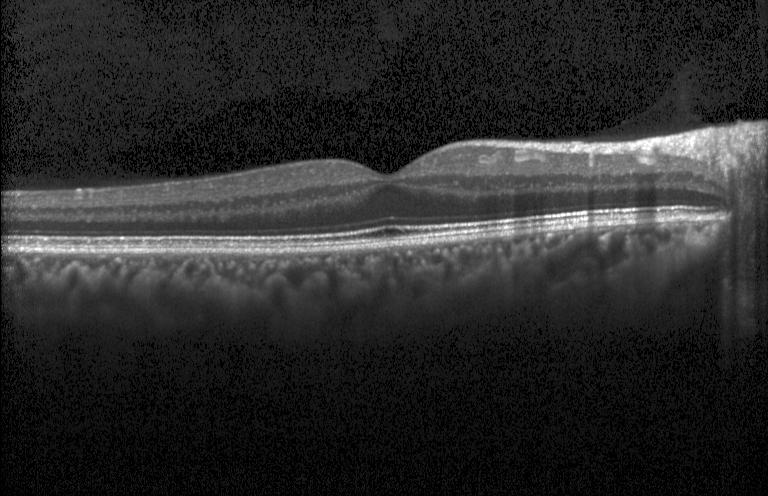

Optical coherence tomography scan — Impression: neither choroidal neovascularization, diabetic macular edema, nor drusen.